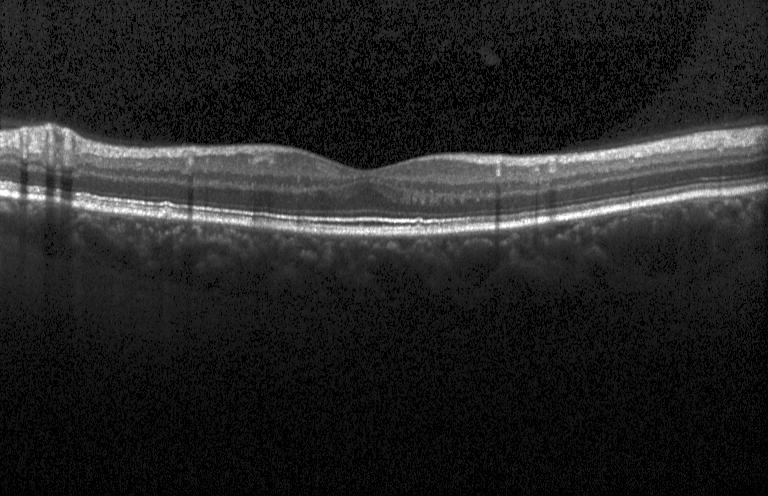

Retinal OCT B-scan
OCT finding: no evidence of CNV, DME, or drusen.